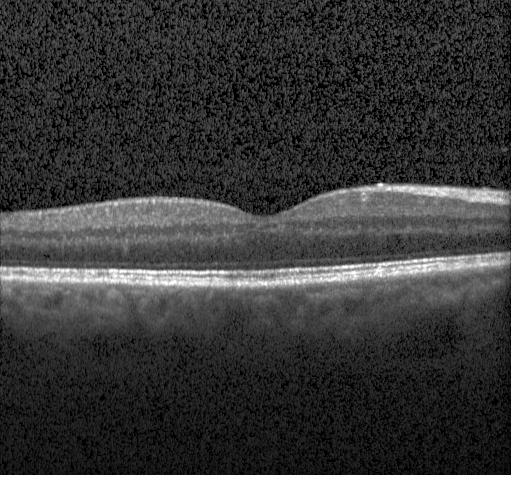
Optical coherence tomography B-scan; instrument: Heidelberg Spectralis; SD-OCT.
Dx: no evidence of CNV, DME, or drusen.